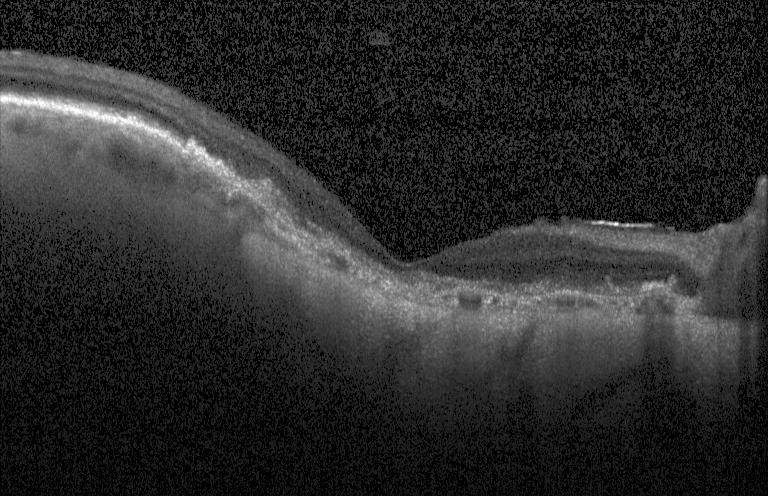

Horizontal scan through the fovea. Optical coherence tomography scan — A choroidal neovascular membrane.